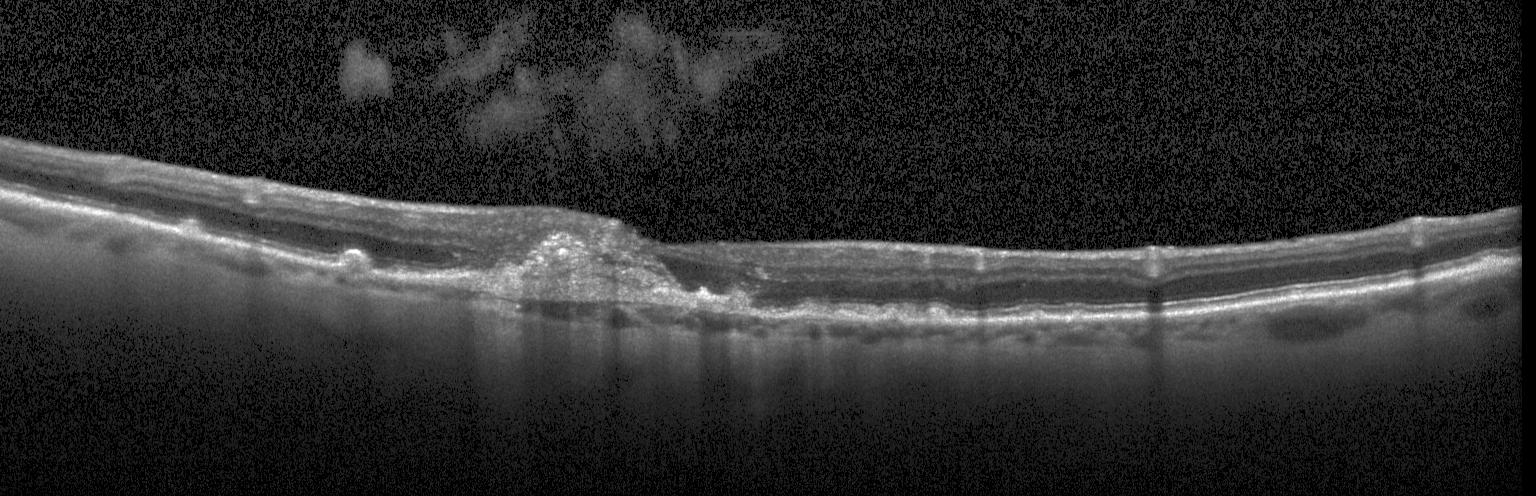 OCT B-scan. Macular scan
Choroidal neovascularization.